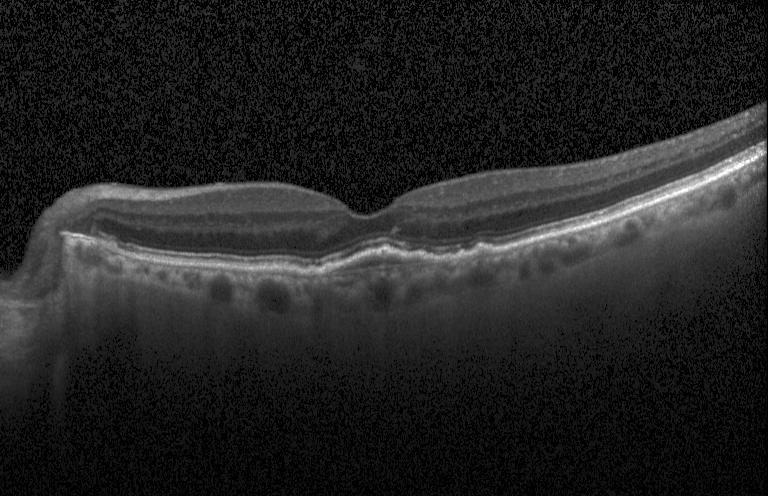

Heidelberg Spectralis OCT system; through the macula; spectral-domain OCT; retinal OCT B-scan — Impression: choroidal neovascularization.